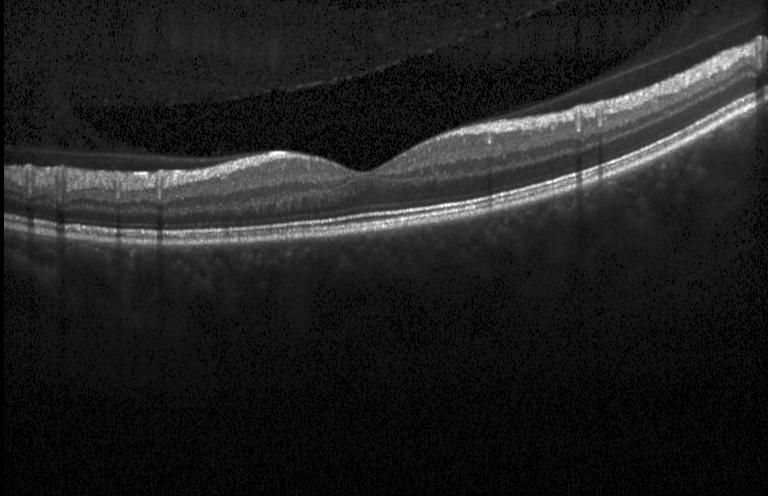
Finding: no choroidal neovascularization, no diabetic macular edema, and no drusen.